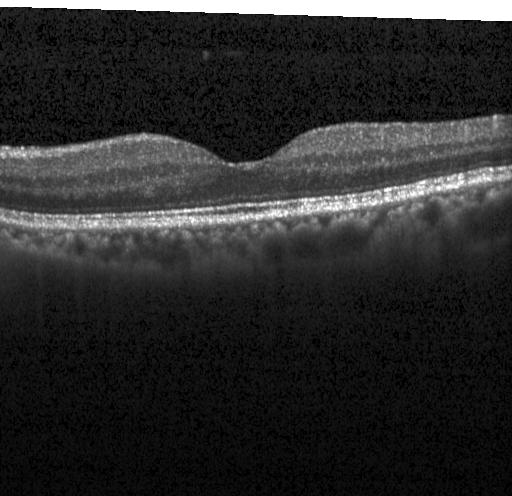

OCT B-scan — Impression: no choroidal neovascularization, no diabetic macular edema, and no drusen.